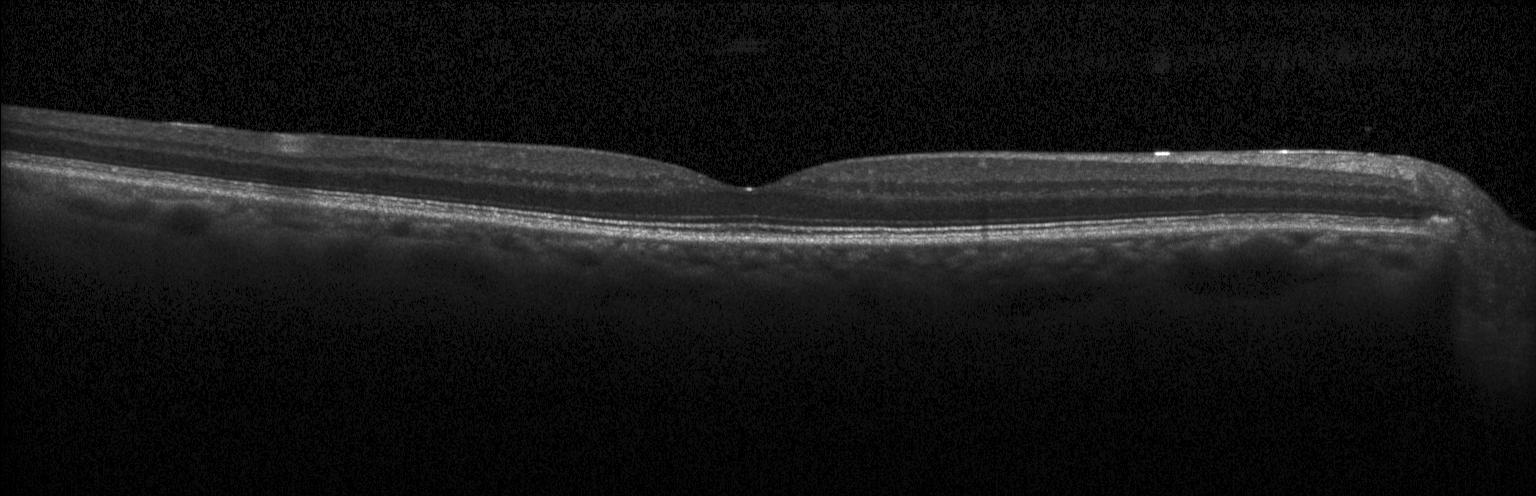 Impression: neither CNV, DME, nor drusen.